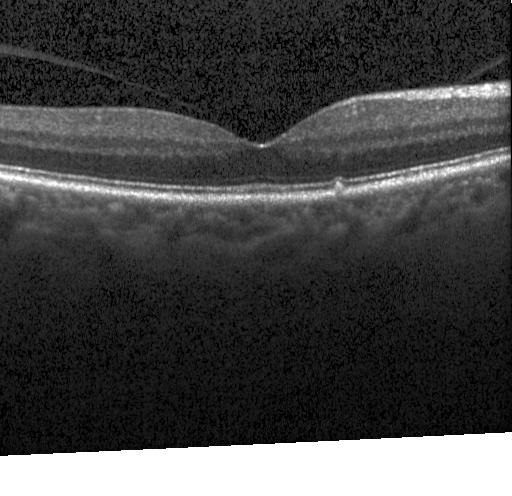
Assessment: multiple drusen.